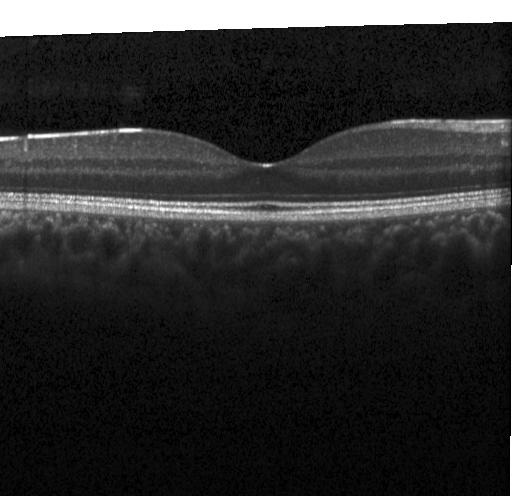
Instrument: Heidelberg Spectralis; SD-OCT; optical coherence tomography scan; fovea-centered
Diagnosis: no choroidal neovascularization, no diabetic macular edema, and no drusen.